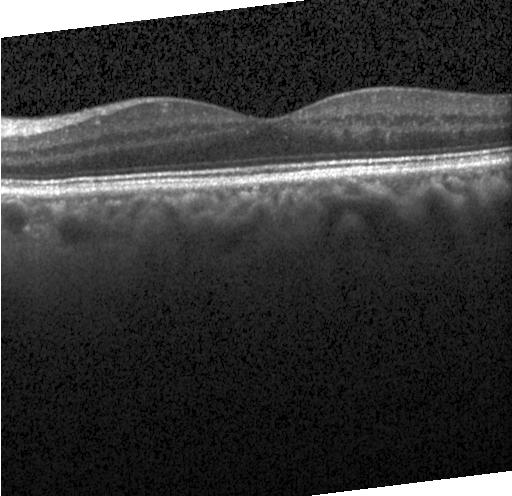
Macular scan, retinal OCT B-scan — This B-scan demonstrates neither choroidal neovascularization, diabetic macular edema, nor drusen.